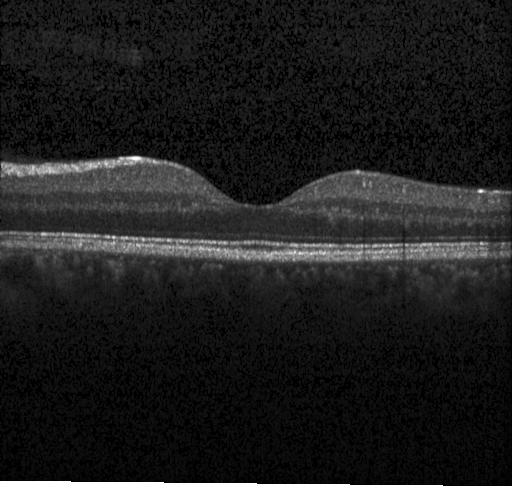

Impression: no choroidal neovascularization, no diabetic macular edema, and no drusen.